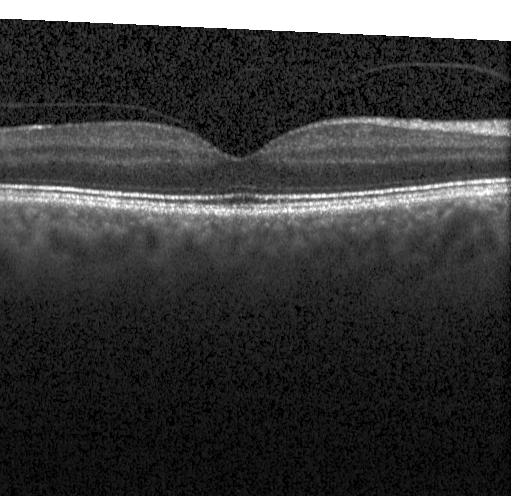
Diagnosis: no choroidal neovascularization, diabetic macular edema, or drusen.